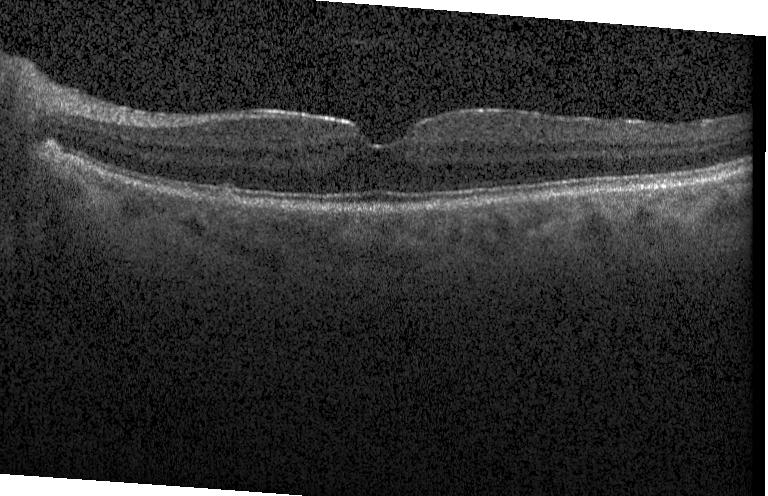

The scan shows no choroidal neovascularization, no diabetic macular edema, and no drusen.